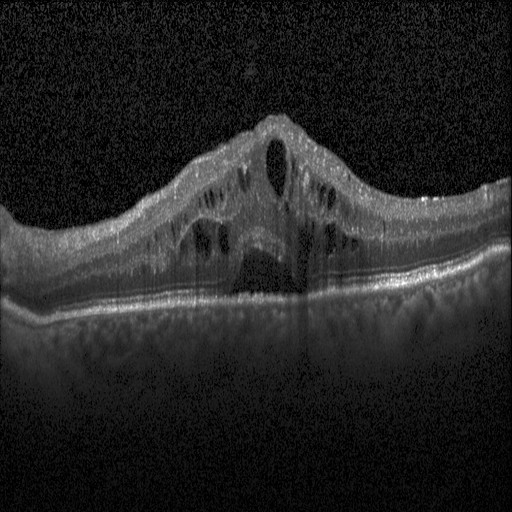 Through the macula. Heidelberg Spectralis OCT system. OCT B-scan. Spectral-domain OCT — Dx: diabetic macular edema (DME).